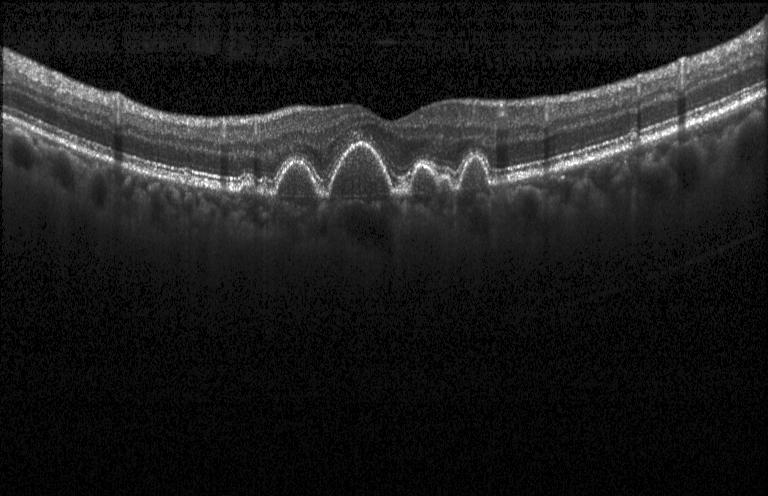

Finding: drusen.